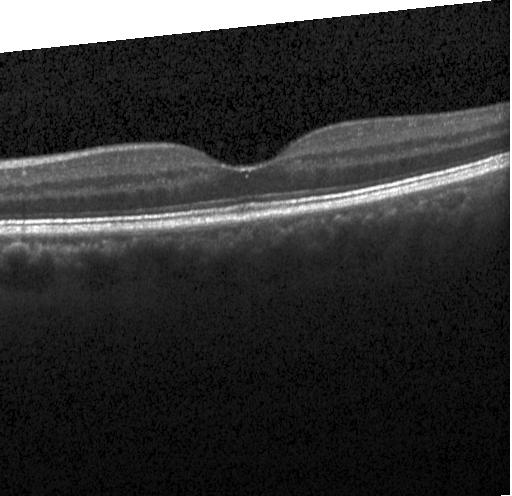 Optical coherence tomography B-scan, spectral-domain optical coherence tomography, Heidelberg Spectralis OCT system, centered on the fovea — Dx: no choroidal neovascularization, no diabetic macular edema, and no drusen.